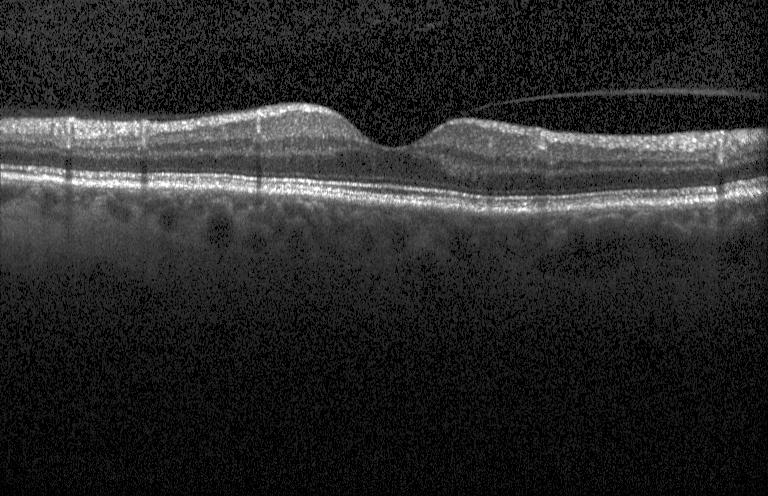
SD-OCT. Heidelberg Spectralis. Fovea-centered. OCT line scan. Finding: no evidence of choroidal neovascularization, diabetic macular edema, or drusen.